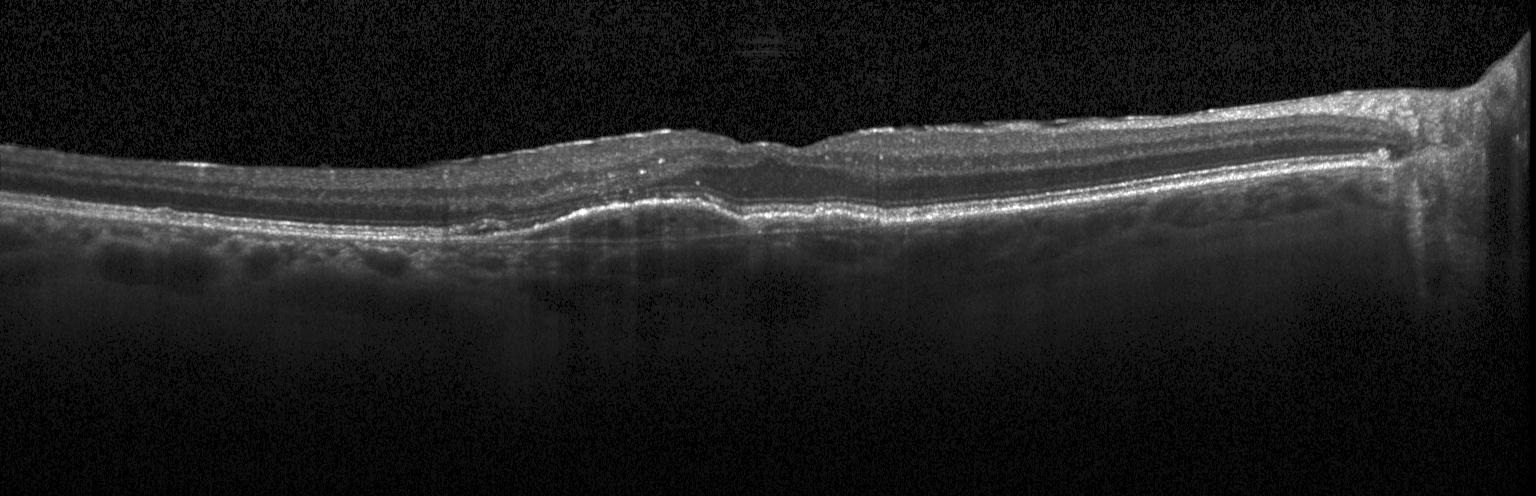

Acquired on a Heidelberg Spectralis · SD-OCT · OCT B-scan. A choroidal neovascular membrane.